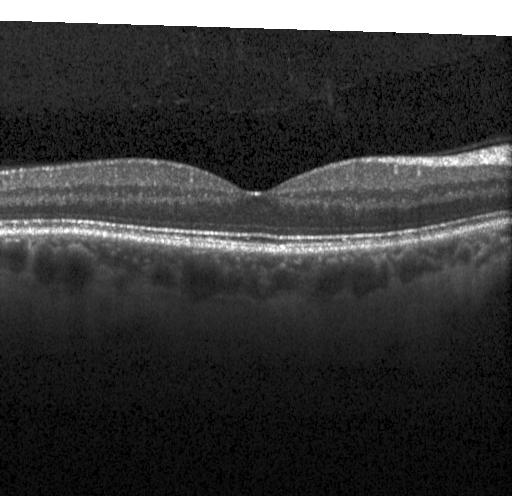
Horizontal scan through the fovea. Retinal OCT B-scan
Impression: no CNV, DME, or drusen.